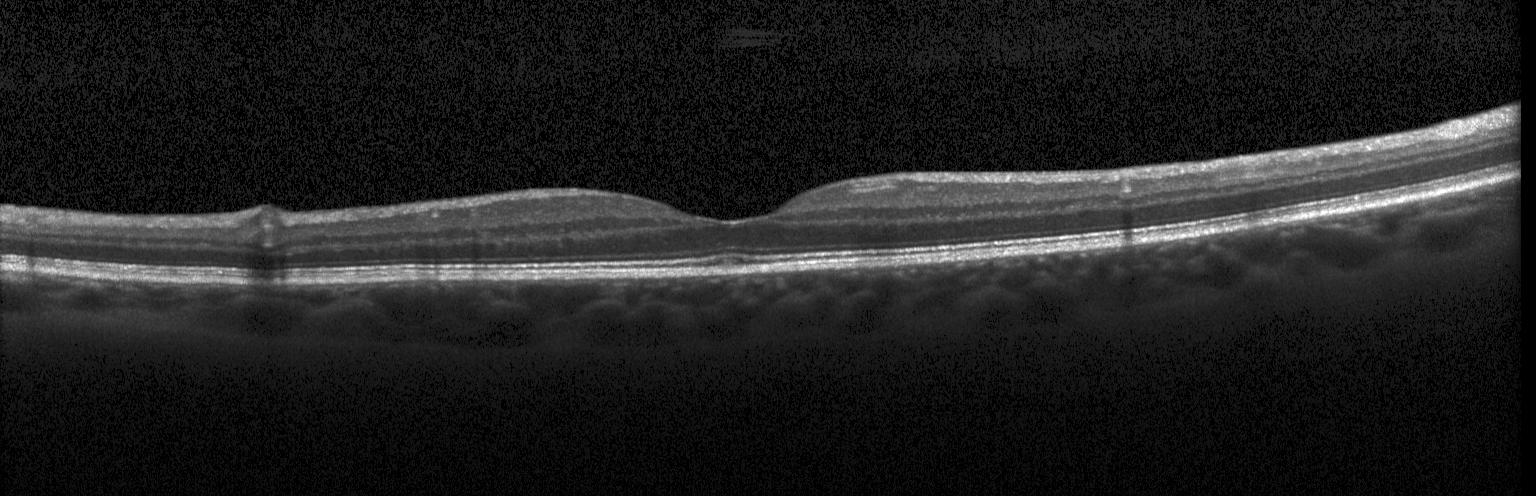
Macular scan. Spectral-domain OCT. OCT B-scan. Acquired on a Heidelberg Spectralis — No evidence of choroidal neovascularization, diabetic macular edema, or drusen.